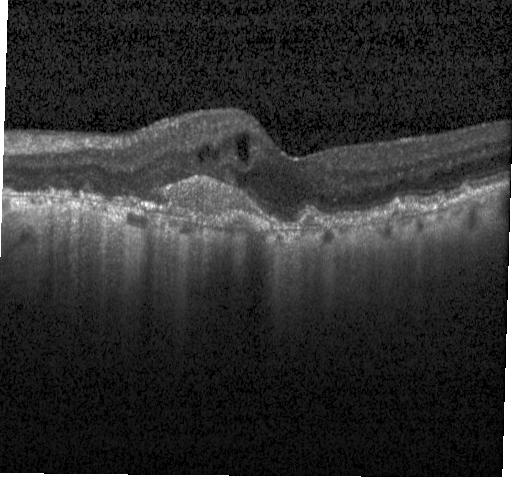

CNV.